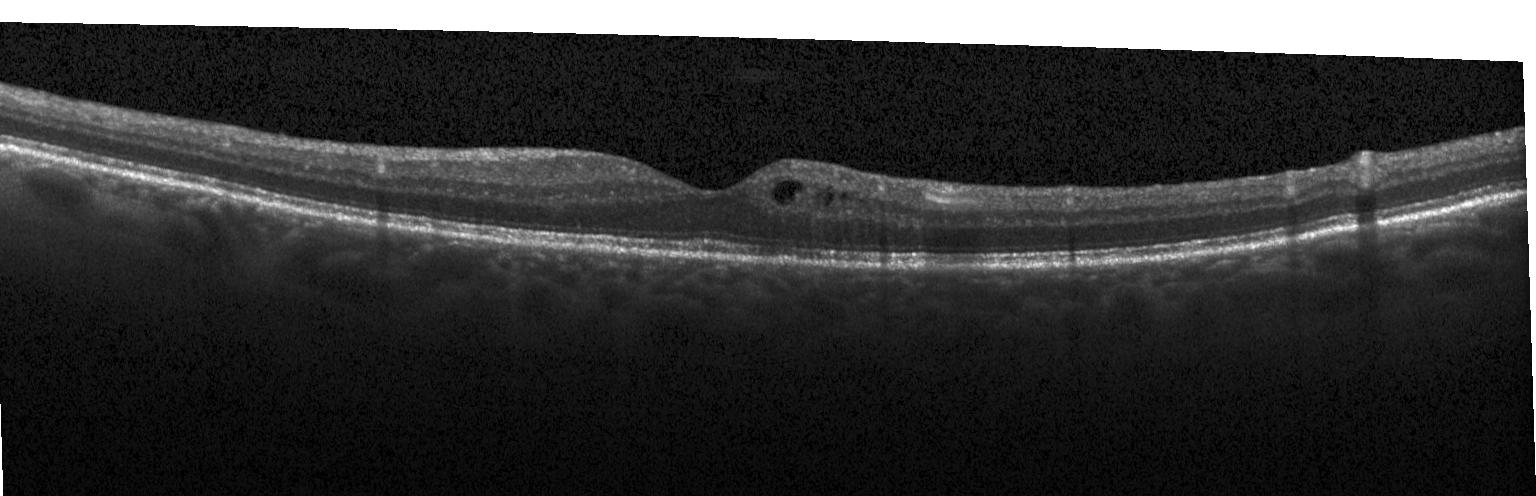
Retinal OCT B-scan.
This B-scan demonstrates diabetic macular edema (DME).